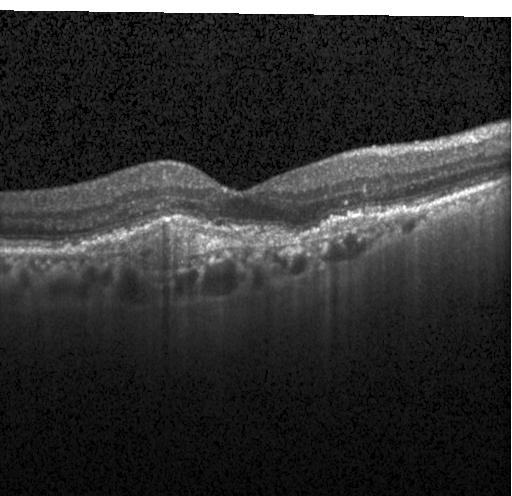
The scan shows a choroidal neovascular membrane.